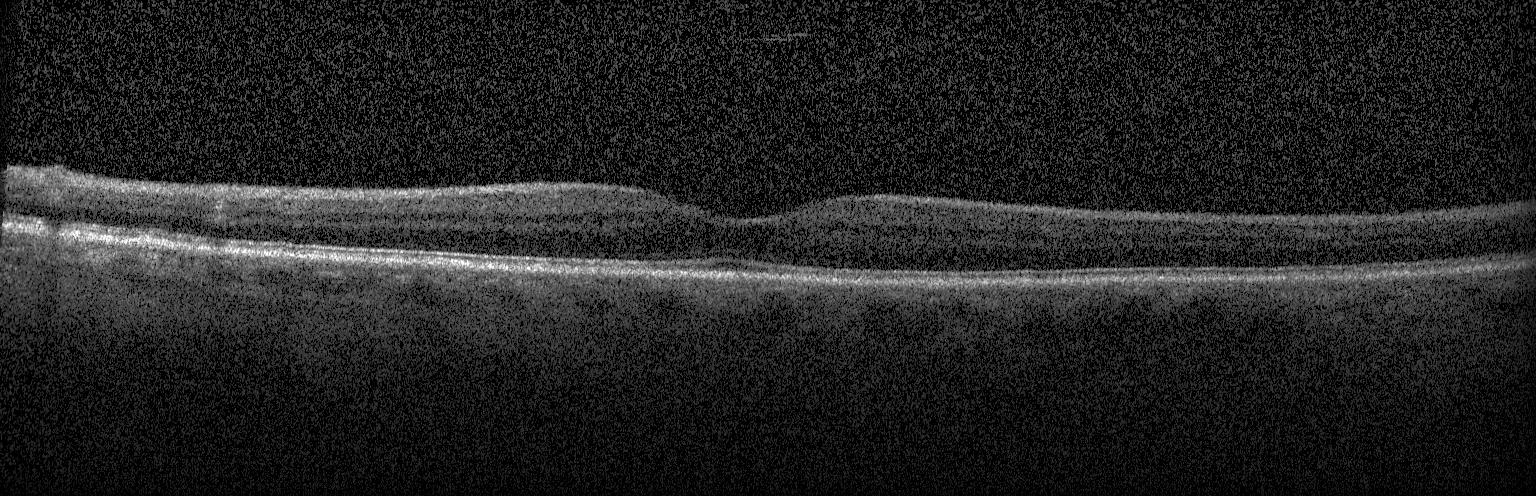
OCT line scan; Heidelberg Spectralis OCT system; horizontal scan through the fovea; SD-OCT.
Impression: no choroidal neovascularization, no diabetic macular edema, and no drusen.